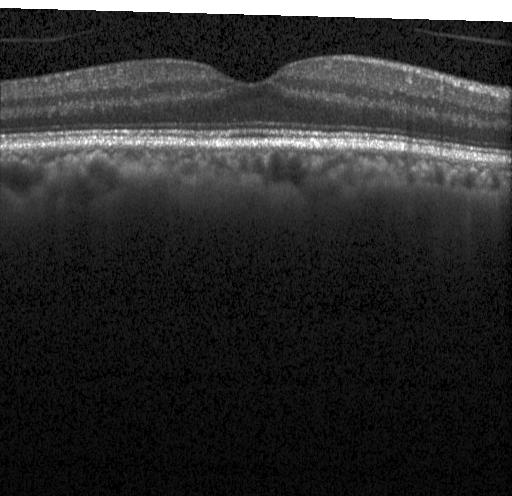

Spectral-domain optical coherence tomography. OCT B-scan.
Impression: neither CNV, DME, nor drusen.